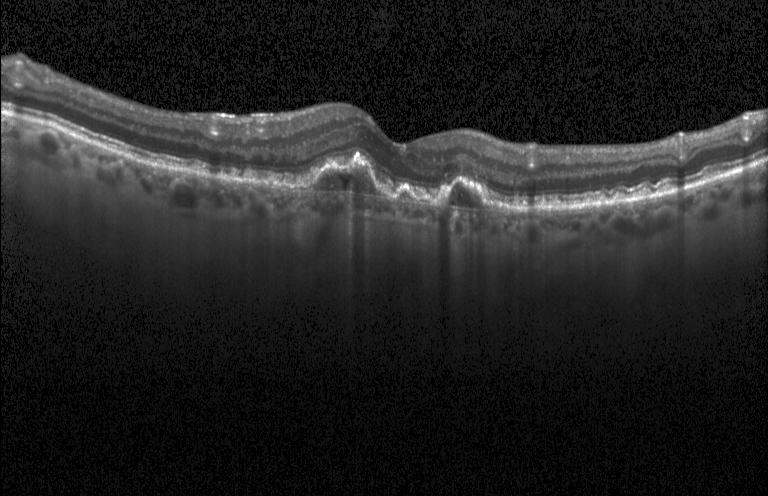

OCT finding: choroidal neovascularization.